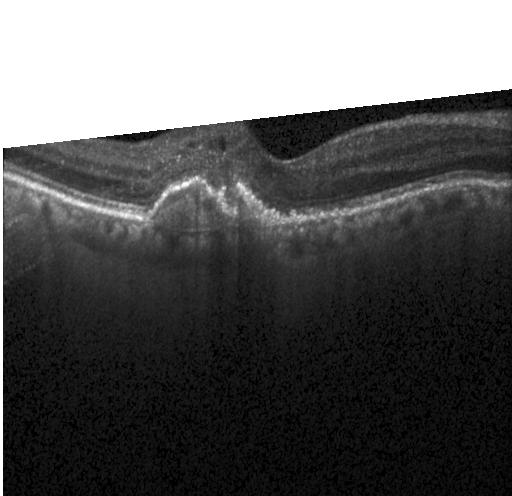

CNV.